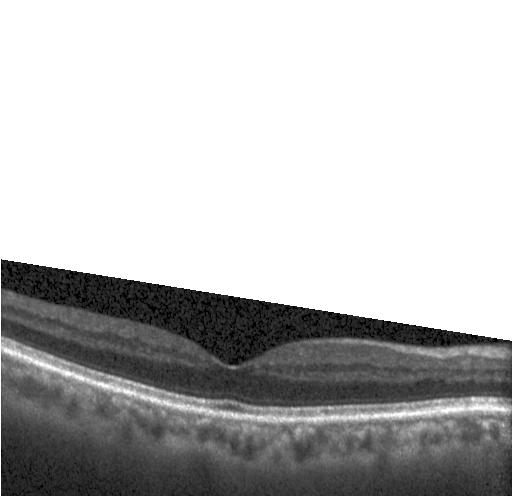

Retinal OCT cross-section
Dx: neither CNV, DME, nor drusen.